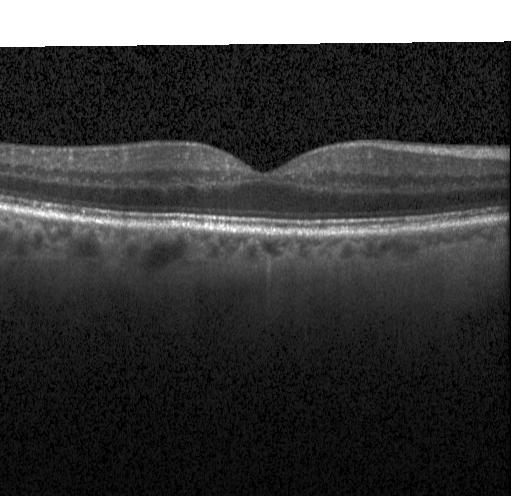 Retinal OCT cross-section showing neither CNV, DME, nor drusen.